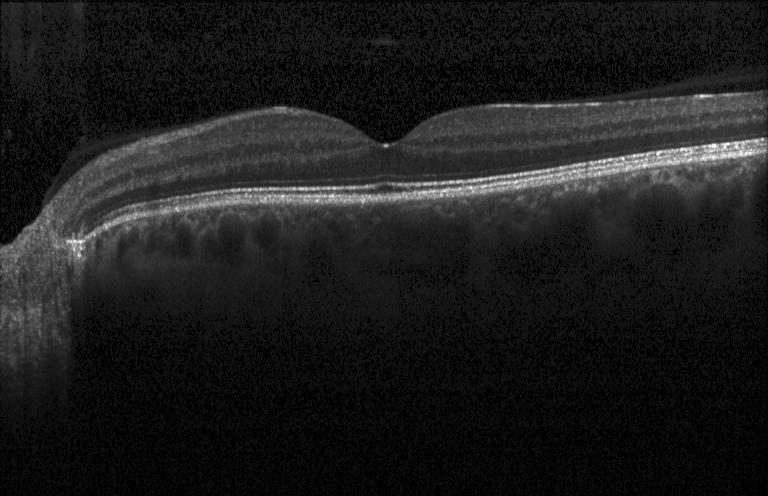 Horizontal scan through the fovea, acquired on a Heidelberg Spectralis, OCT B-scan
Assessment: no choroidal neovascularization, no diabetic macular edema, and no drusen.